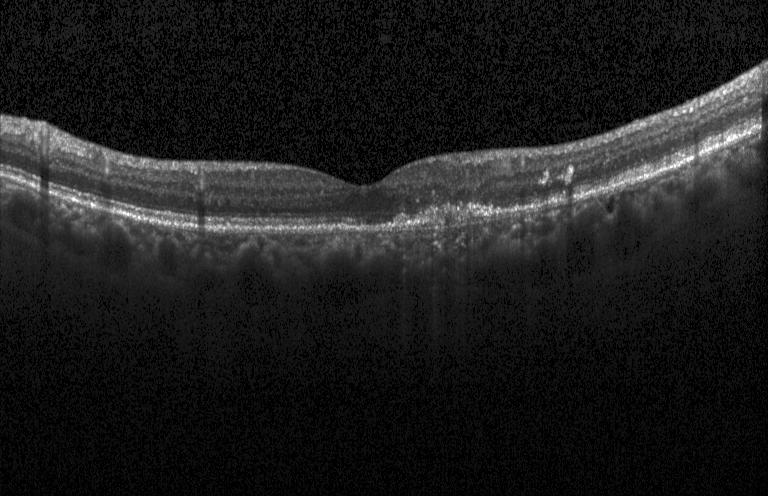
OCT finding: CNV.